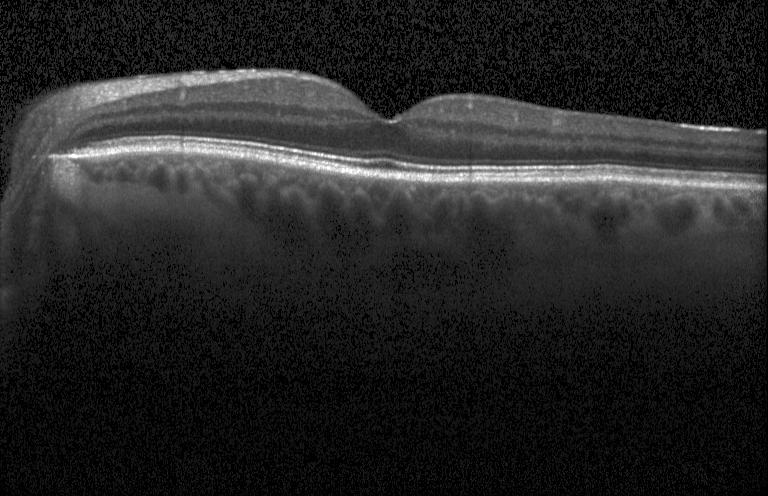 Retinal OCT B-scan. Spectral-domain optical coherence tomography. Diagnosis: no CNV, DME, or drusen.